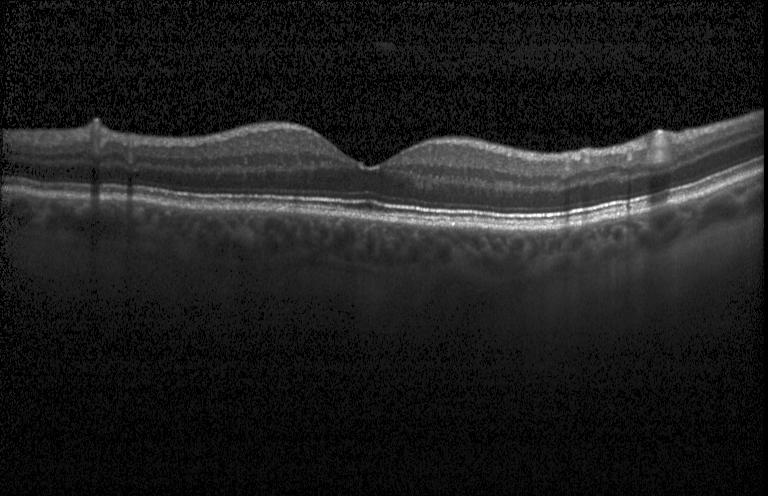 OCT B-scan
The scan shows no evidence of choroidal neovascularization, diabetic macular edema, or drusen.